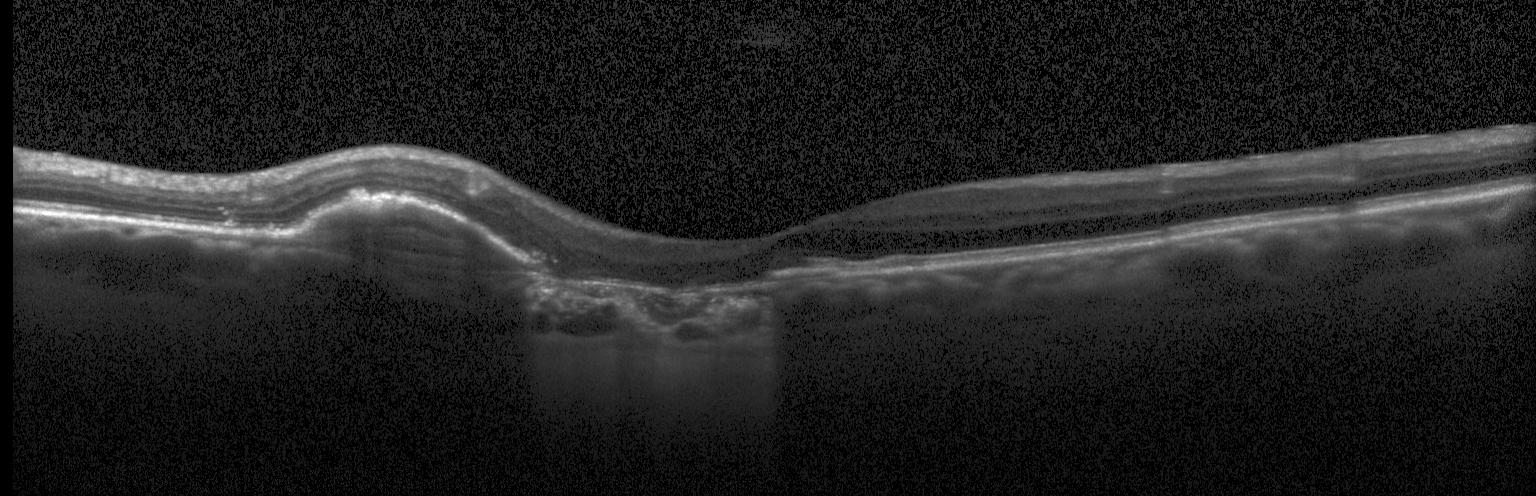 OCT B-scan showing a choroidal neovascular membrane.